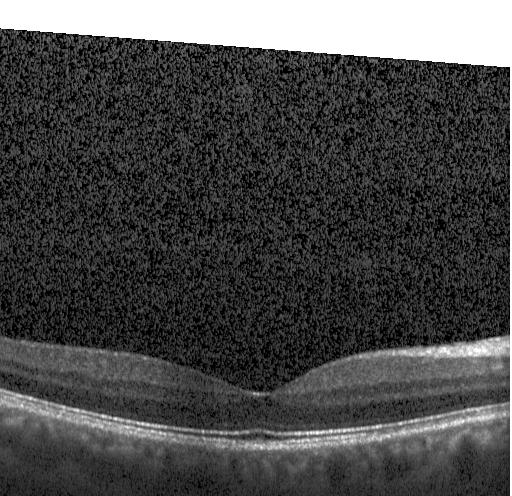

SD-OCT; OCT B-scan; through the macula; acquired on a Heidelberg Spectralis. No evidence of CNV, DME, or drusen.